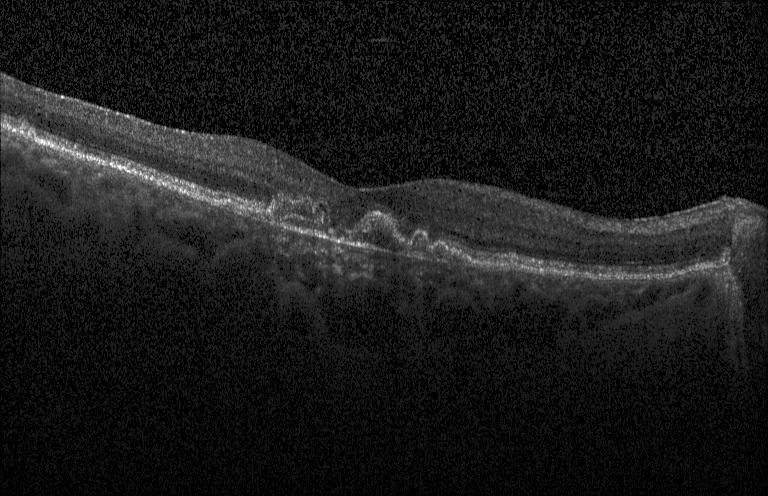

Retinal OCT cross-section
Impression: a choroidal neovascular membrane.